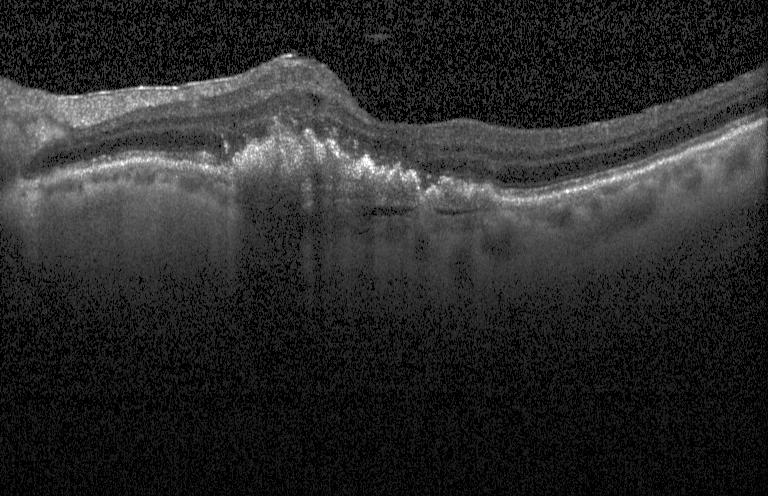

Optical coherence tomography scan · centered on the fovea · Heidelberg Spectralis. Impression: choroidal neovascularization (CNV).